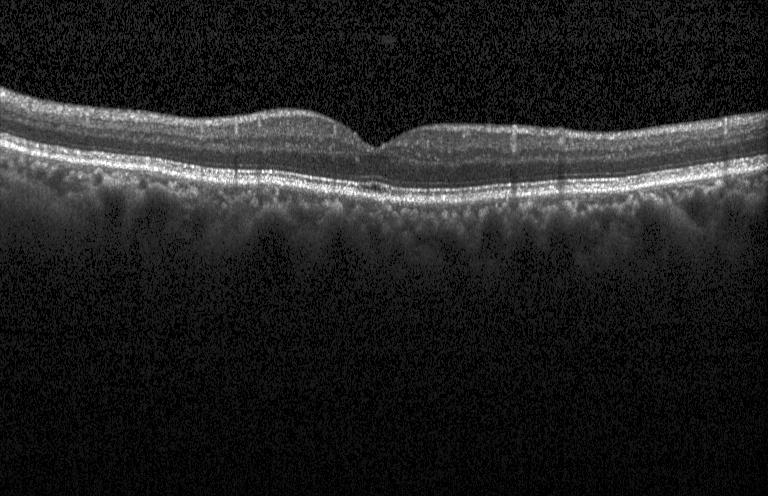 Retinal OCT B-scan. Macular OCT: no choroidal neovascularization, diabetic macular edema, or drusen.